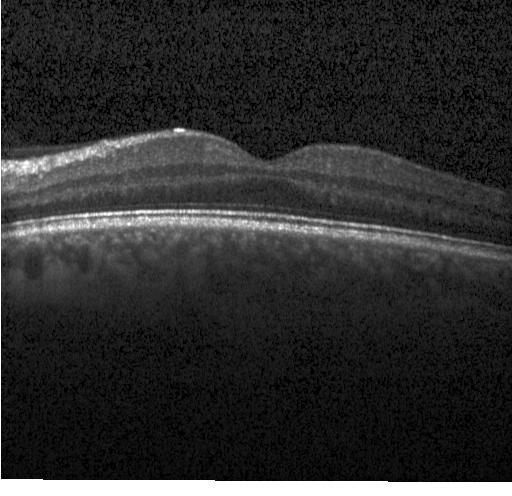 OCT B-scan showing neither choroidal neovascularization, diabetic macular edema, nor drusen.